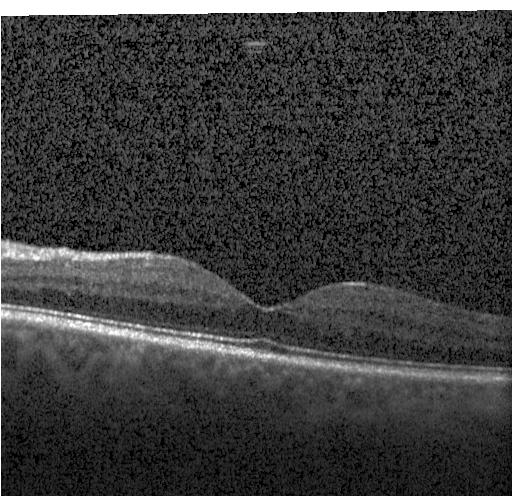 Through the macula; optical coherence tomography B-scan; spectral-domain optical coherence tomography
This B-scan demonstrates no CNV, DME, or drusen.